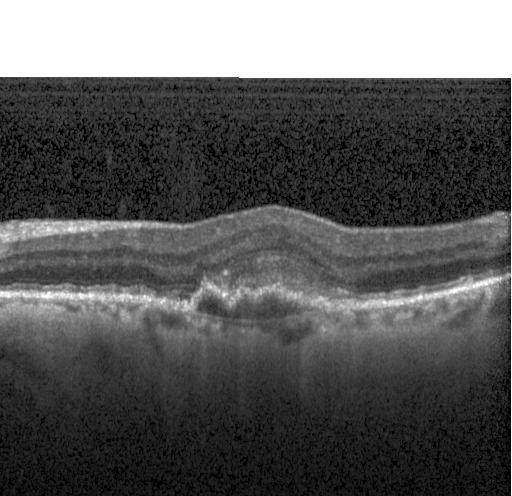
Finding: a choroidal neovascular membrane.